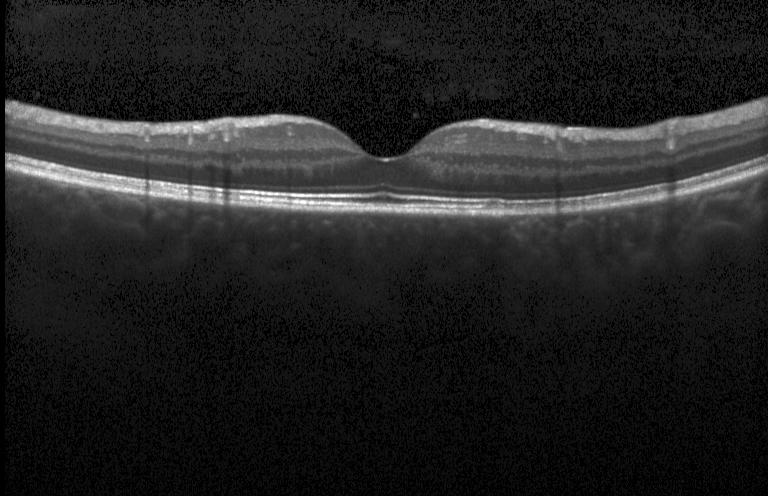

OCT B-scan
Macular OCT: no evidence of choroidal neovascularization, diabetic macular edema, or drusen.